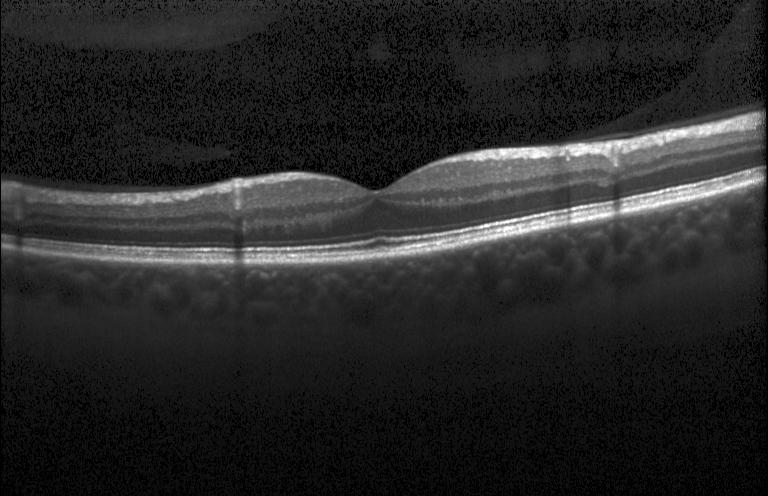 OCT finding: no CNV, no DME, and no drusen.